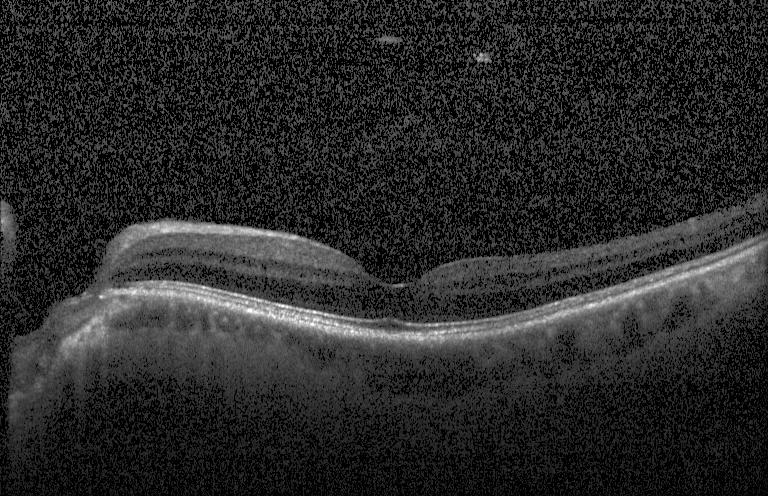
Spectral-domain optical coherence tomography; acquired on a Heidelberg Spectralis; retinal OCT B-scan.
No evidence of CNV, DME, or drusen.